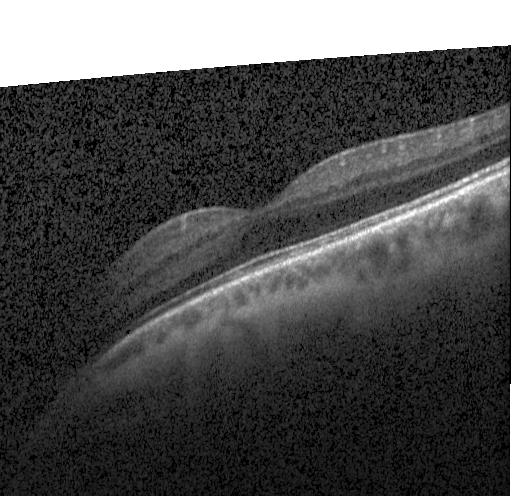
Spectral-domain OCT B-scan: no CNV, no DME, and no drusen.